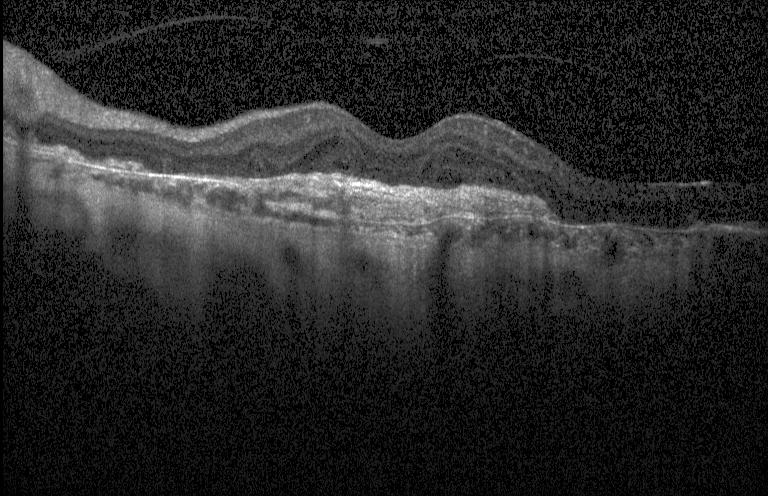

Finding: CNV.